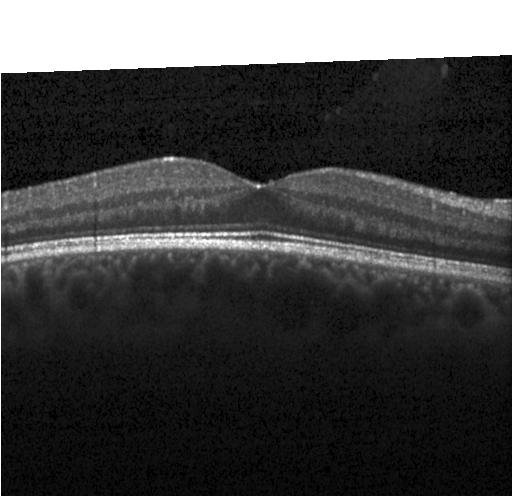

Dx: no choroidal neovascularization, diabetic macular edema, or drusen.